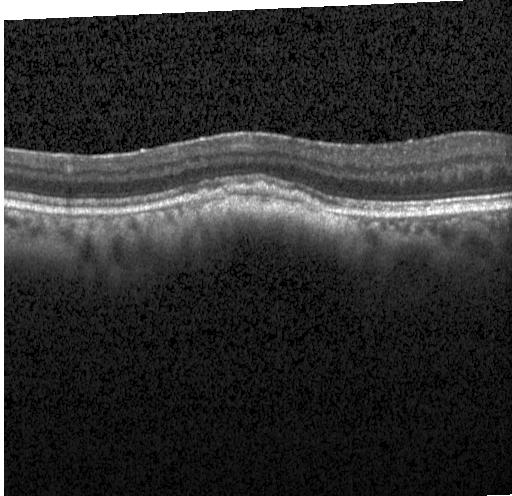 The scan shows a choroidal neovascular membrane.